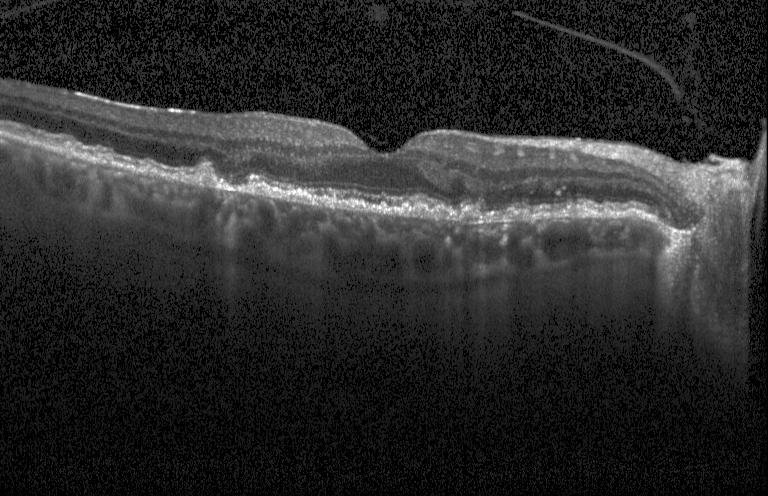

Impression: multiple drusen.